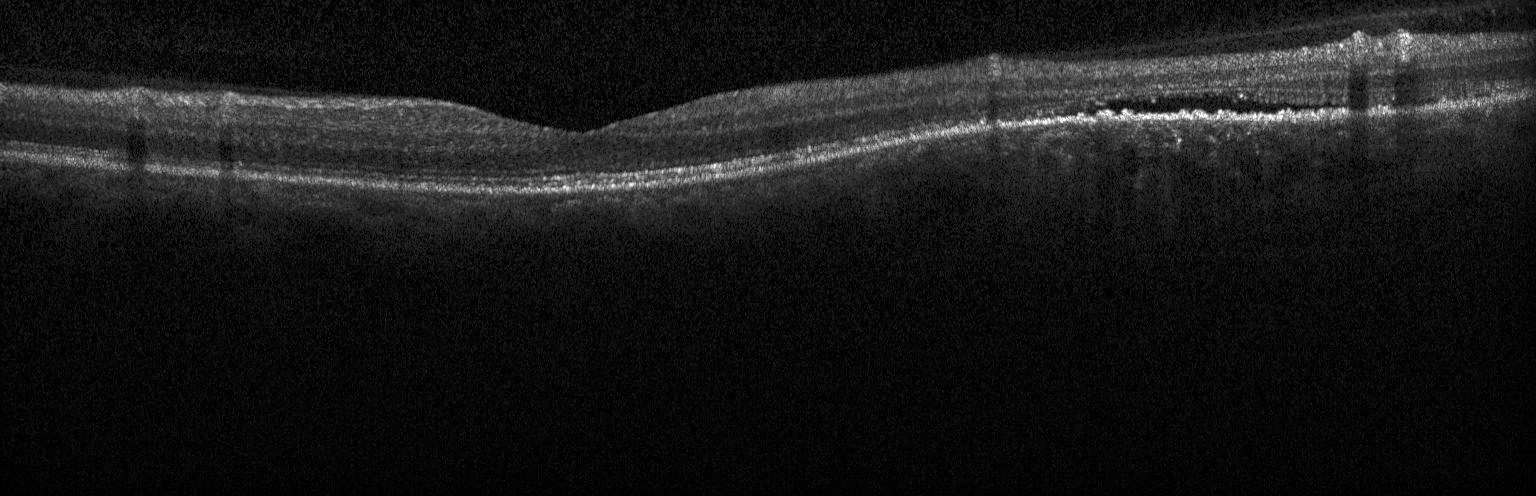
Finding: CNV.